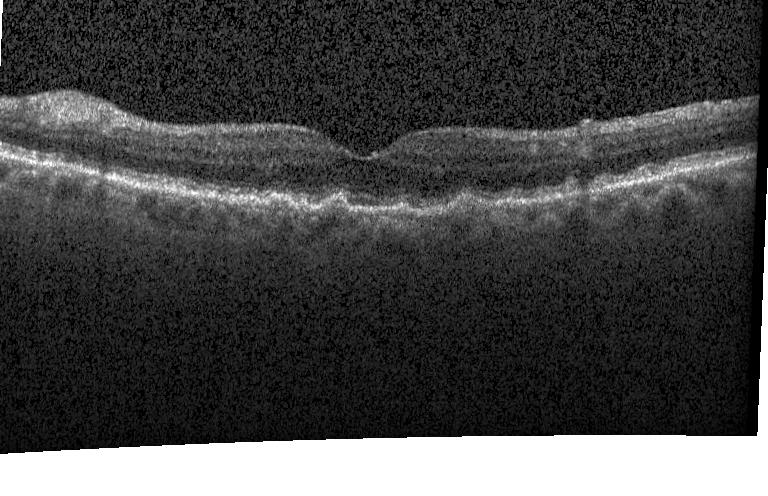 Optical coherence tomography scan. Horizontal scan through the fovea. Instrument: Heidelberg Spectralis. SD-OCT
Multiple drusen.